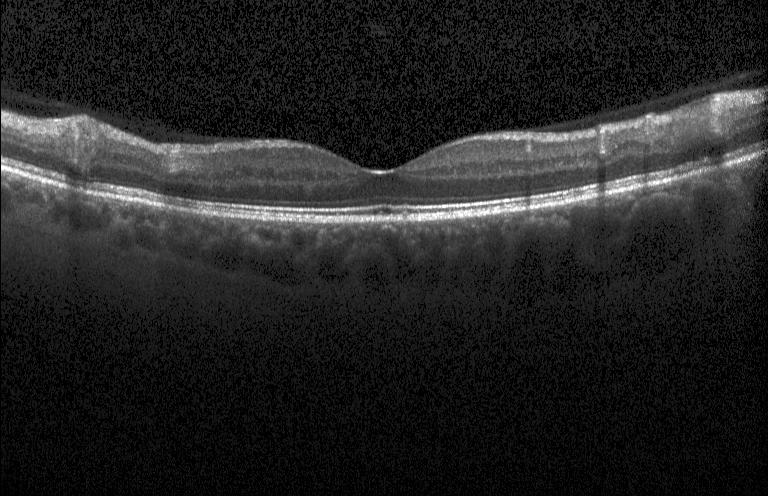 Optical coherence tomography scan — OCT finding: no choroidal neovascularization, no diabetic macular edema, and no drusen.